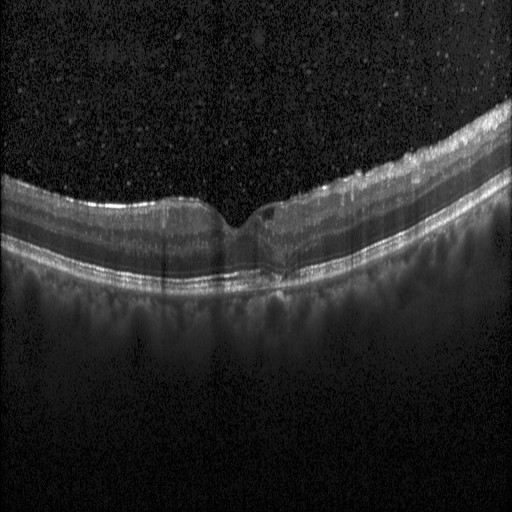 Heidelberg Spectralis OCT system · SD-OCT · fovea-centered · optical coherence tomography scan. Impression: DME.